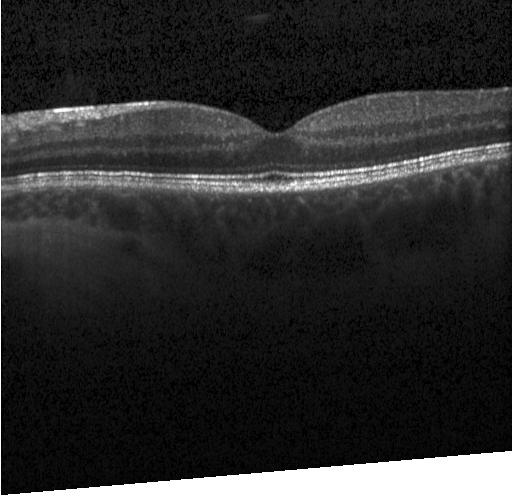

Macular OCT: neither choroidal neovascularization, diabetic macular edema, nor drusen.